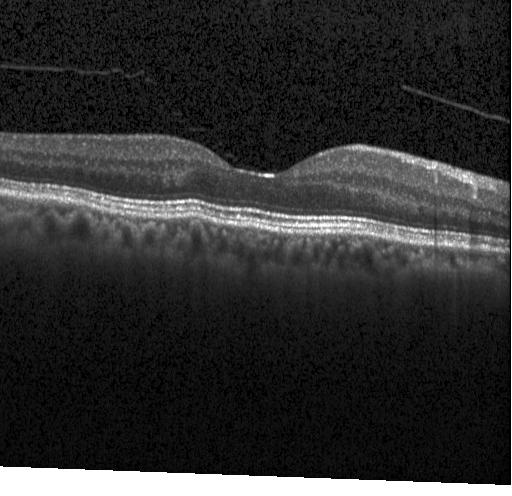
OCT finding: no CNV, no DME, and no drusen.